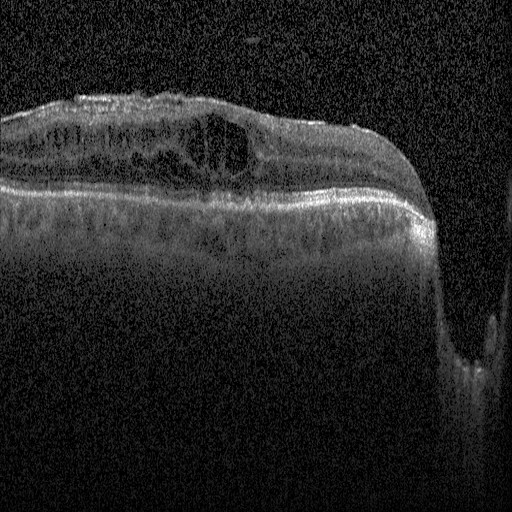 Through the macula, optical coherence tomography B-scan — Impression: DME.